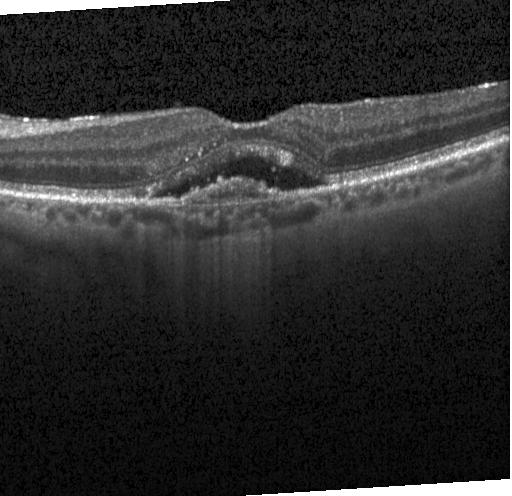
Diagnosis: a choroidal neovascular membrane.